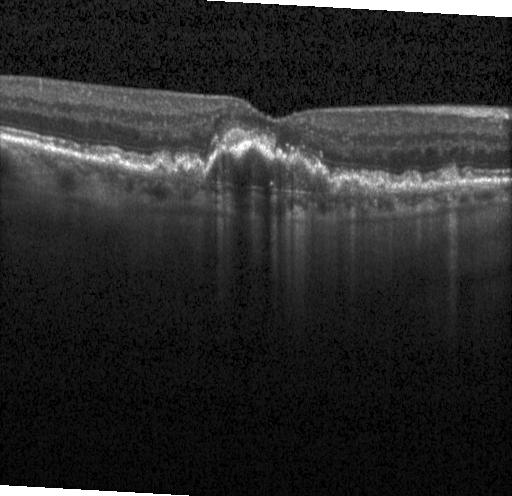
Impression: choroidal neovascularization.